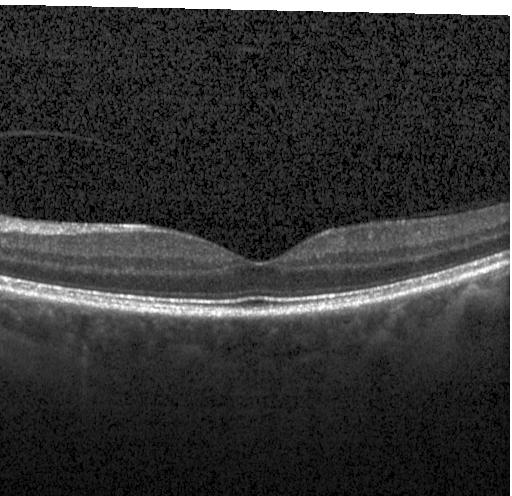 Centered on the fovea · optical coherence tomography B-scan · acquired on a Heidelberg Spectralis.
Finding: no choroidal neovascularization, no diabetic macular edema, and no drusen.